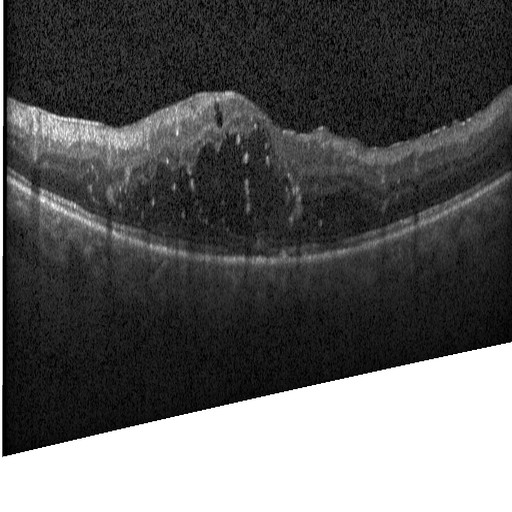
SD-OCT. Retinal OCT B-scan. Centered on the fovea
Diagnosis: diabetic macular edema (DME).